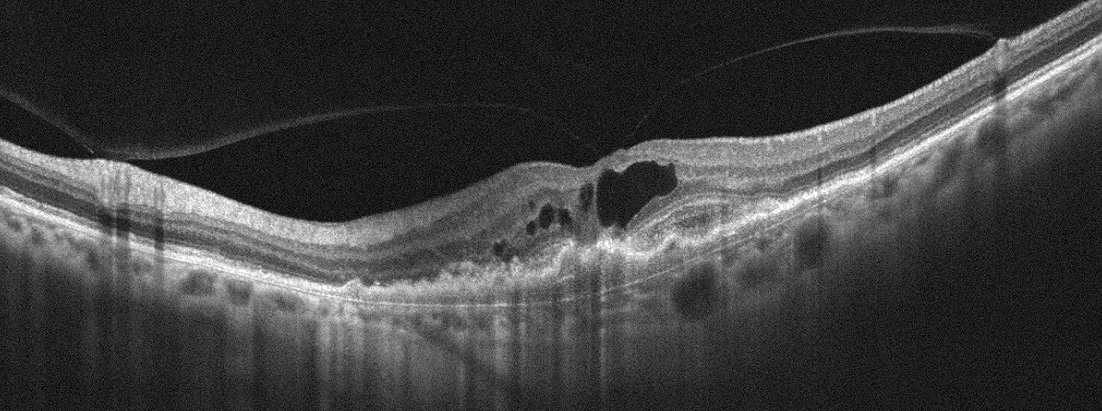 Optical coherence tomography scan
Macular OCT: age-related macular degeneration (AMD).